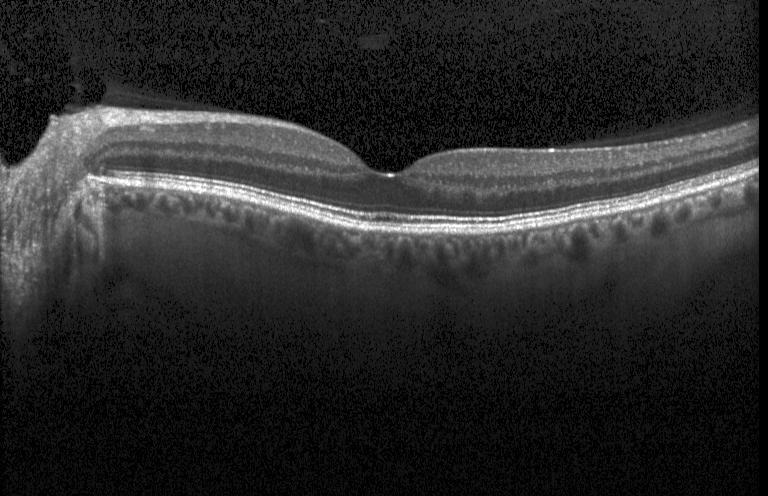

Impression: no choroidal neovascularization, diabetic macular edema, or drusen.